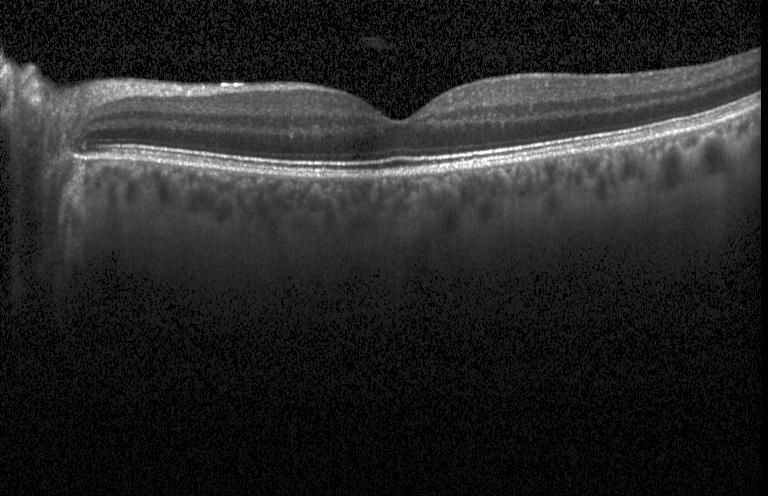

Macular scan, Heidelberg Spectralis, retinal OCT B-scan
Diagnosis: no CNV, DME, or drusen.